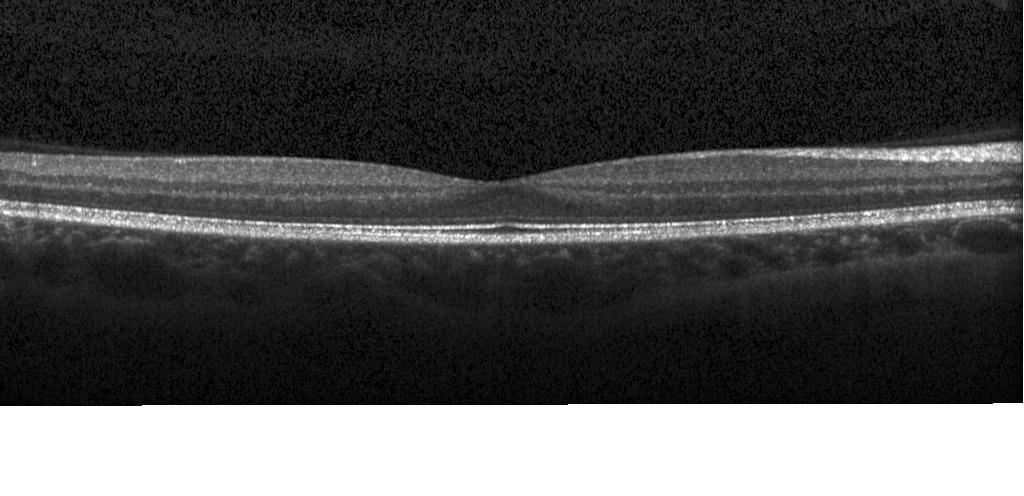
Spectral-domain optical coherence tomography; horizontal scan through the fovea; retinal OCT cross-section
Dx: no CNV, DME, or drusen.